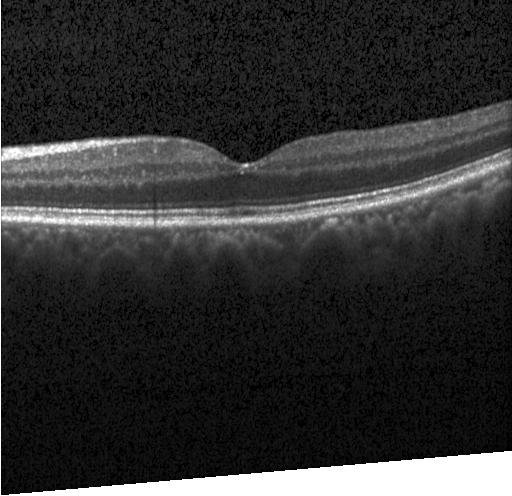 OCT B-scan — Assessment: neither choroidal neovascularization, diabetic macular edema, nor drusen.